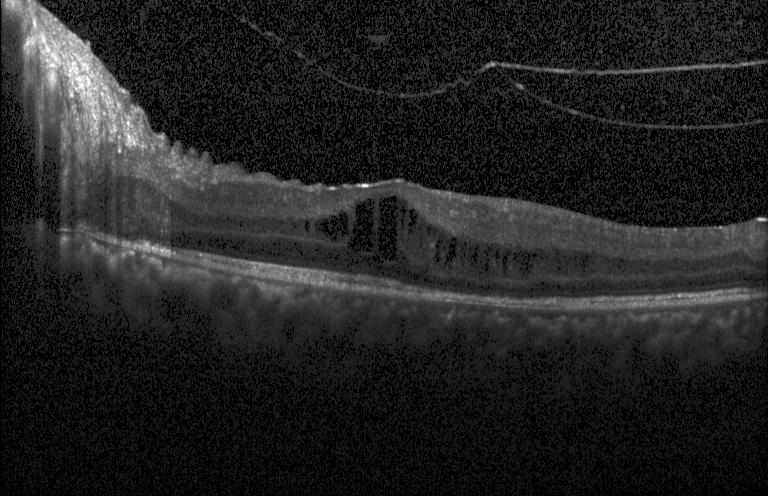
Spectral-domain OCT B-scan: diabetic macular edema (DME).